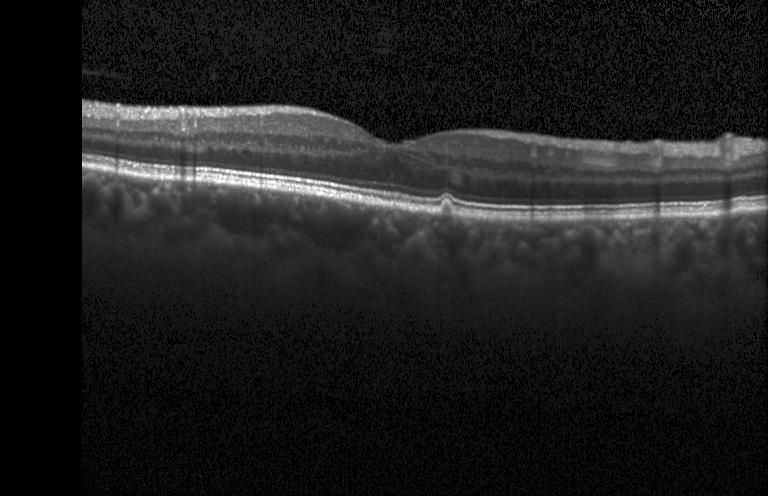

Macular OCT demonstrating sub-RPE drusenoid deposits.